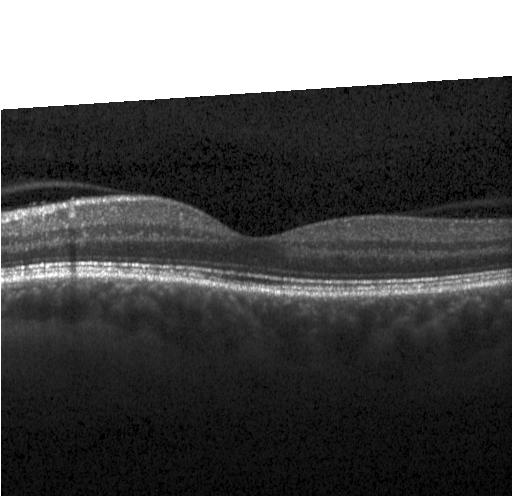 OCT B-scan
Diagnosis: no choroidal neovascularization, diabetic macular edema, or drusen.